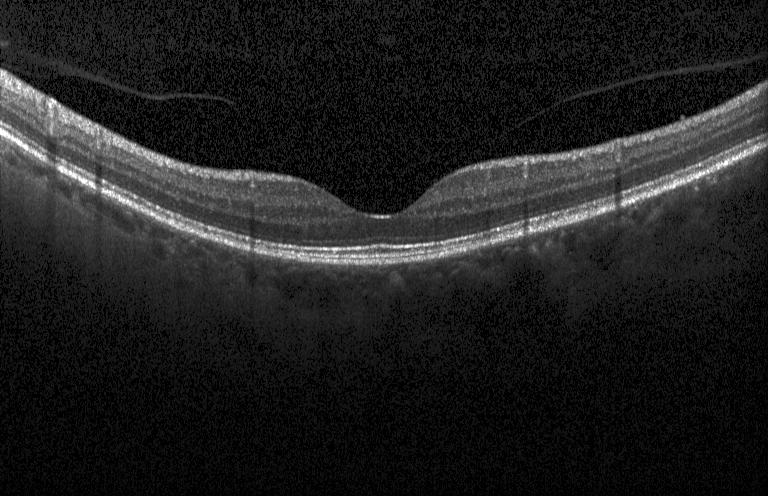 Macular OCT: no choroidal neovascularization, diabetic macular edema, or drusen.